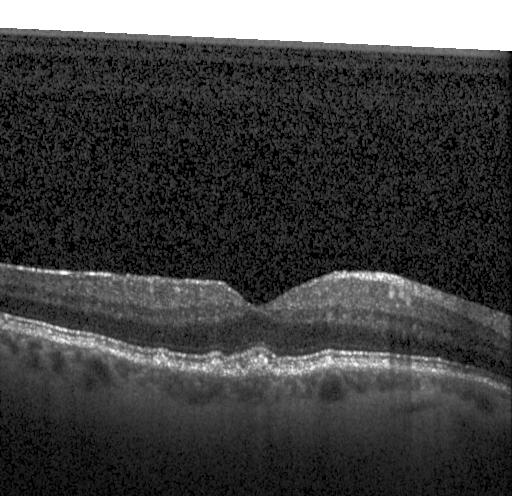 Heidelberg Spectralis OCT system · SD-OCT · centered on the fovea · OCT B-scan — OCT finding: drusen.